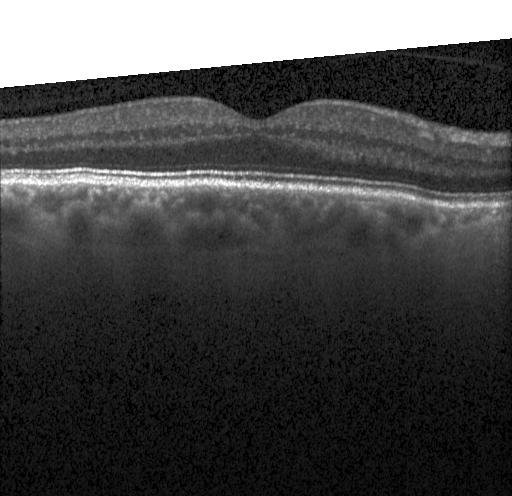
OCT finding: no evidence of choroidal neovascularization, diabetic macular edema, or drusen.